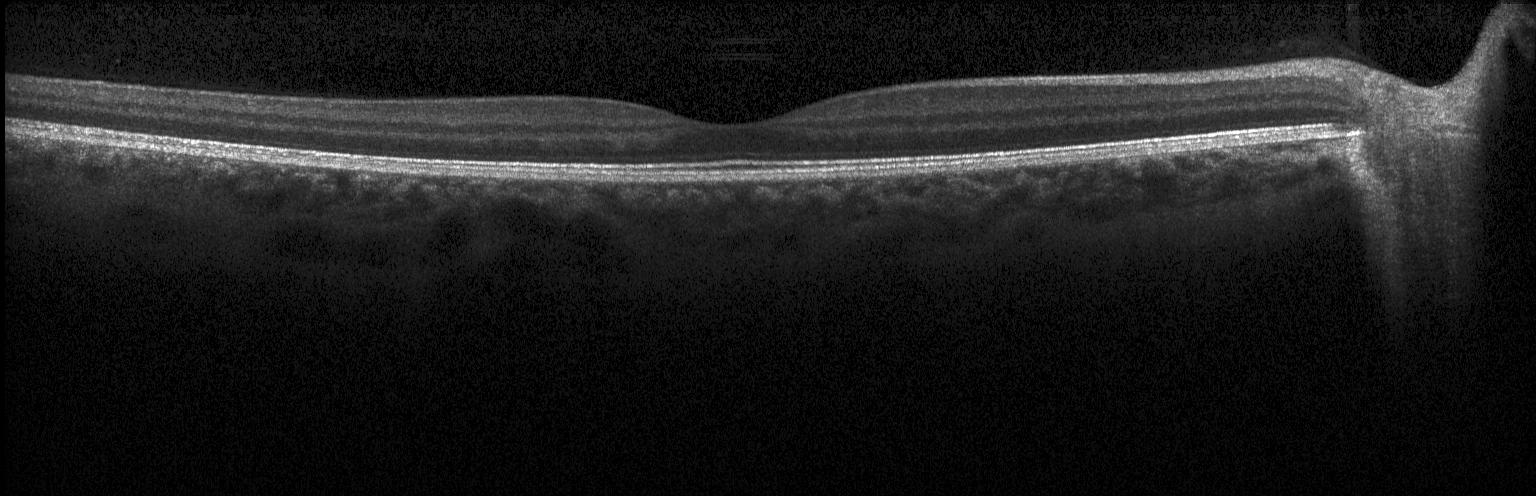
Retinal OCT B-scan — Dx: neither CNV, DME, nor drusen.